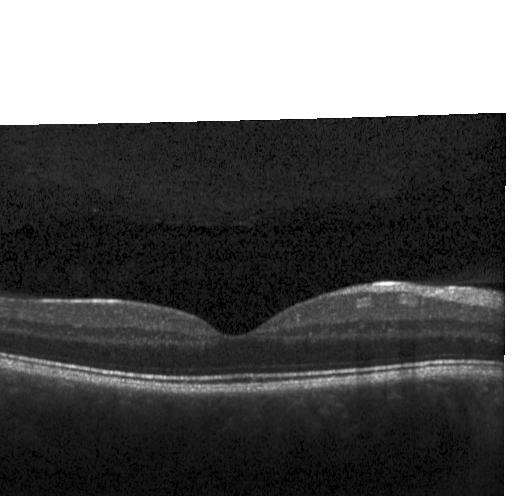

Acquired on a Heidelberg Spectralis. Spectral-domain optical coherence tomography. Through the macula. Optical coherence tomography scan. Dx: no CNV, DME, or drusen.